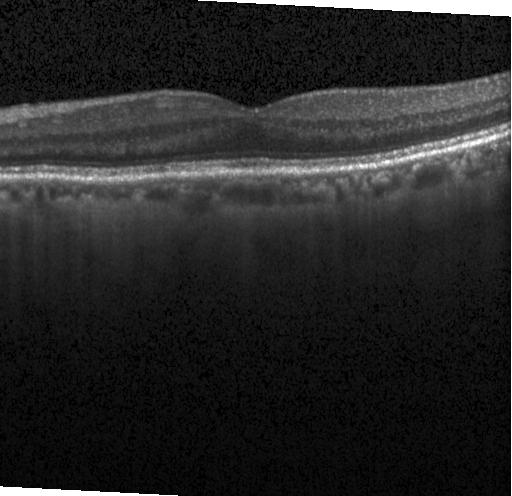

Through the macula. Optical coherence tomography B-scan. Impression: neither CNV, DME, nor drusen.